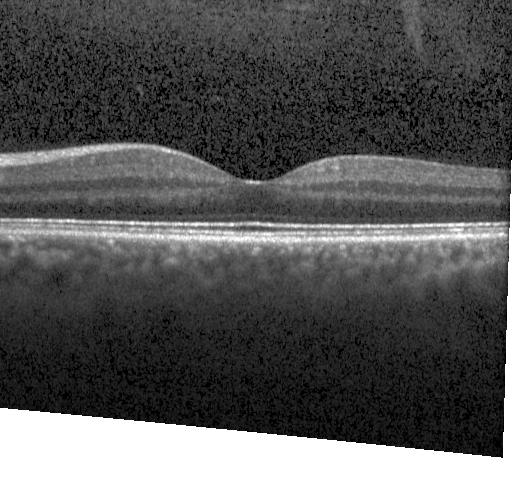 Finding: no evidence of choroidal neovascularization, diabetic macular edema, or drusen.